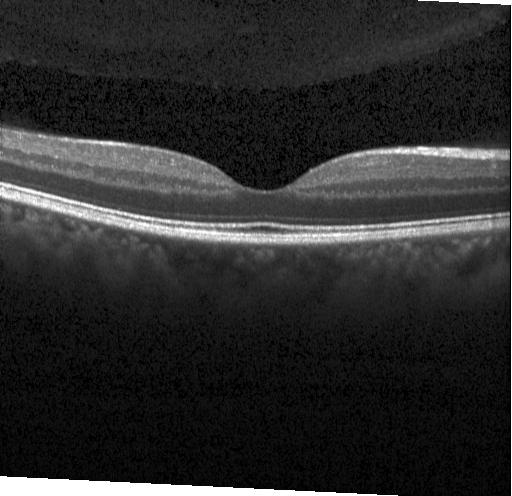 Retinal OCT cross-section — Diagnosis: no choroidal neovascularization, diabetic macular edema, or drusen.